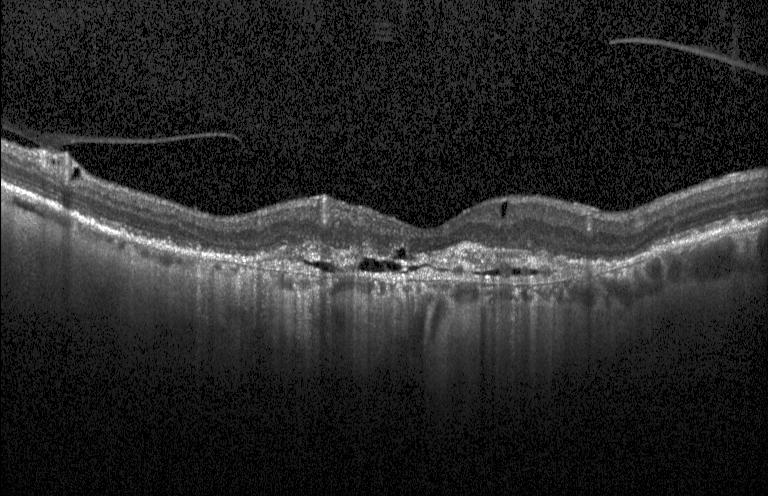 Optical coherence tomography scan, Heidelberg Spectralis OCT system, through the macula — Diagnosis: choroidal neovascularization.